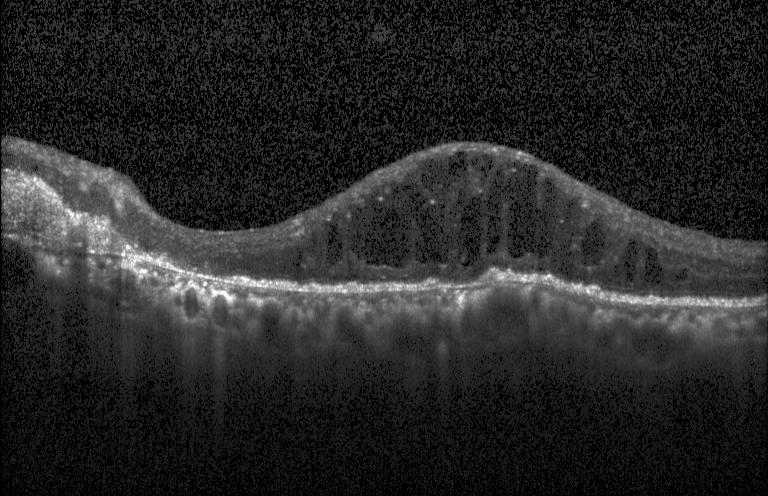 A choroidal neovascular membrane.